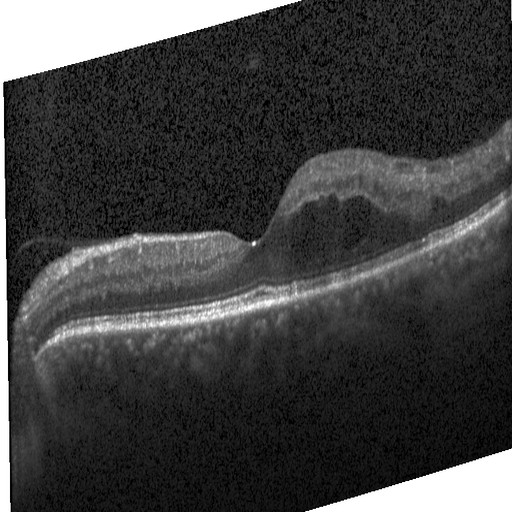 OCT B-scan. Assessment: diabetic macular edema (DME).